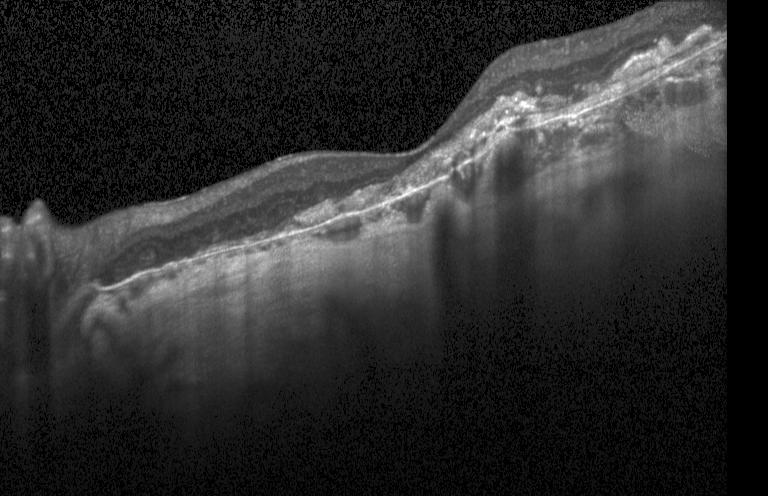 OCT line scan. Through the macula. Spectral-domain OCT. Impression: choroidal neovascularization (CNV).